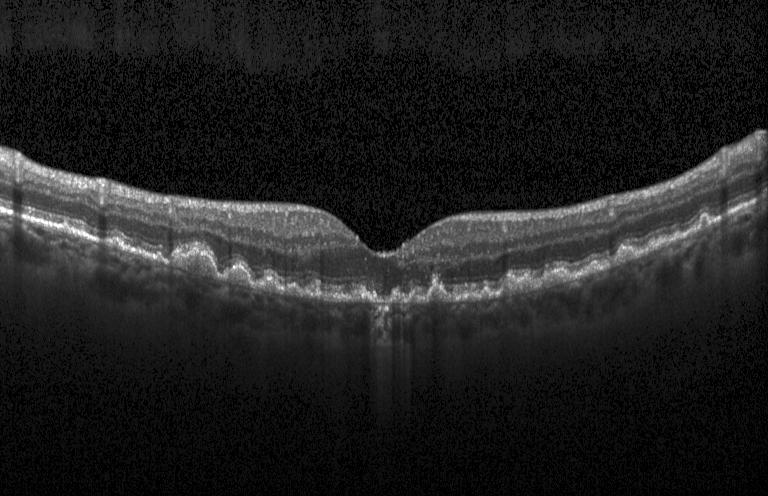
This B-scan demonstrates drusen.